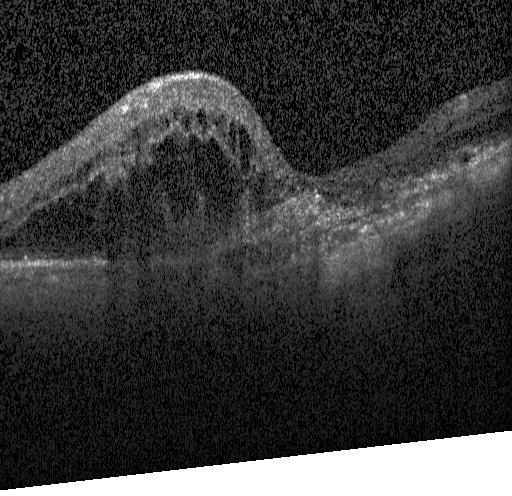
OCT line scan — The scan shows a choroidal neovascular membrane.